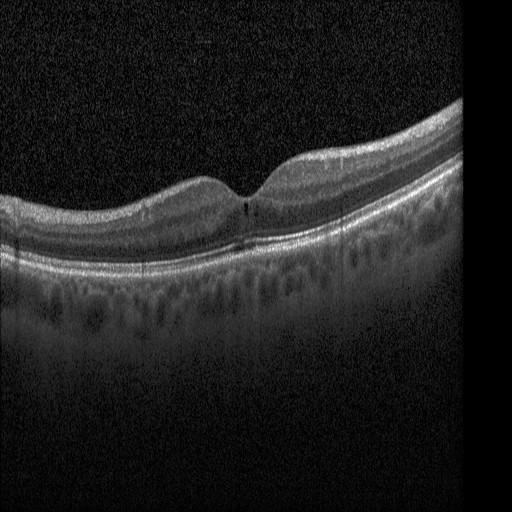
Horizontal scan through the fovea, optical coherence tomography B-scan, acquired on a Heidelberg Spectralis, spectral-domain optical coherence tomography — This B-scan demonstrates DME.